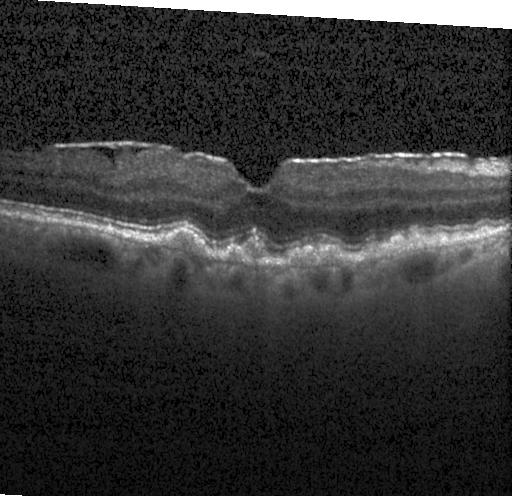 OCT scan showing multiple drusen.